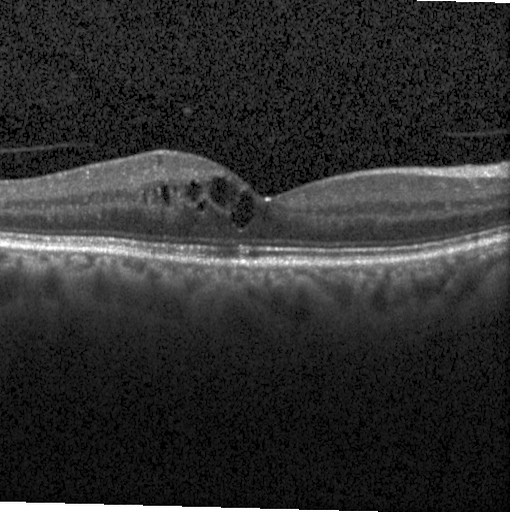
OCT line scan
Macular OCT: diabetic macular edema (DME).